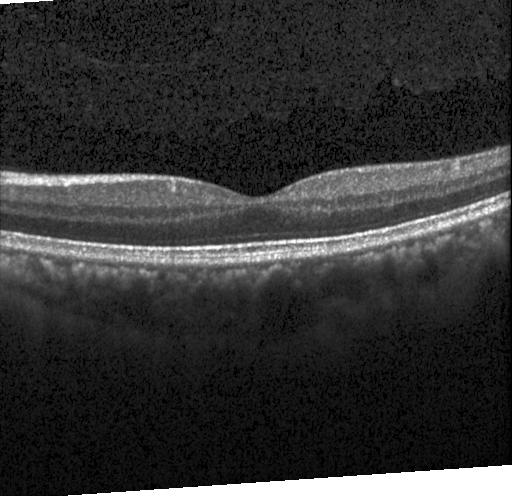 Instrument: Heidelberg Spectralis · spectral-domain optical coherence tomography · centered on the fovea · retinal OCT B-scan — This B-scan demonstrates neither CNV, DME, nor drusen.